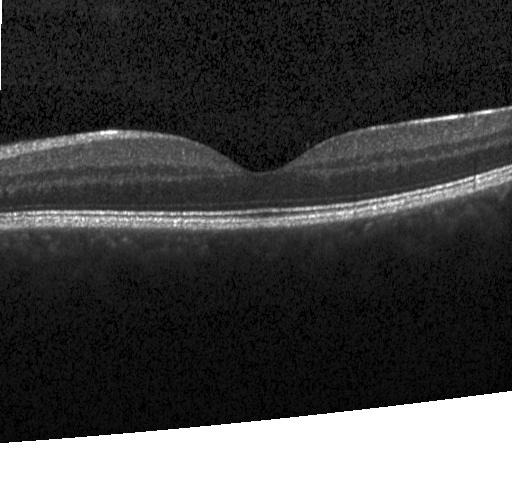
Assessment: no CNV, DME, or drusen.